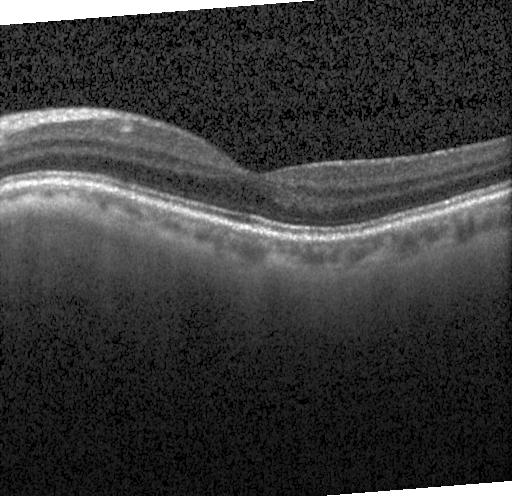 Assessment: no choroidal neovascularization, diabetic macular edema, or drusen.